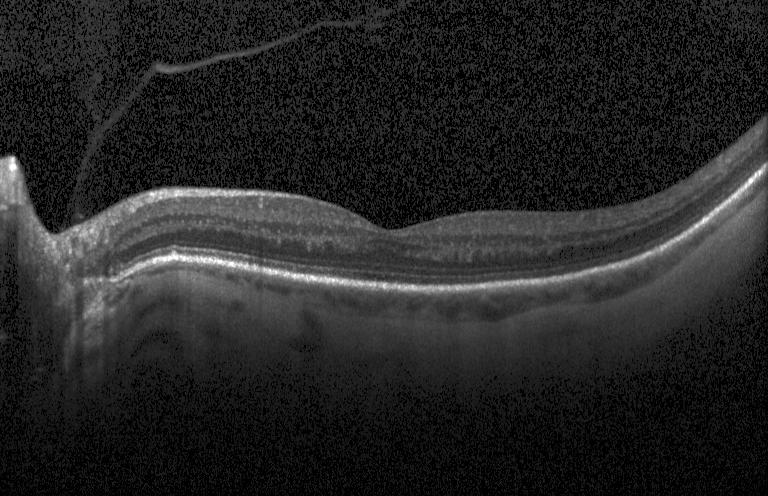 Spectral-domain optical coherence tomography. Optical coherence tomography scan. Macular scan. Finding: neither choroidal neovascularization, diabetic macular edema, nor drusen.